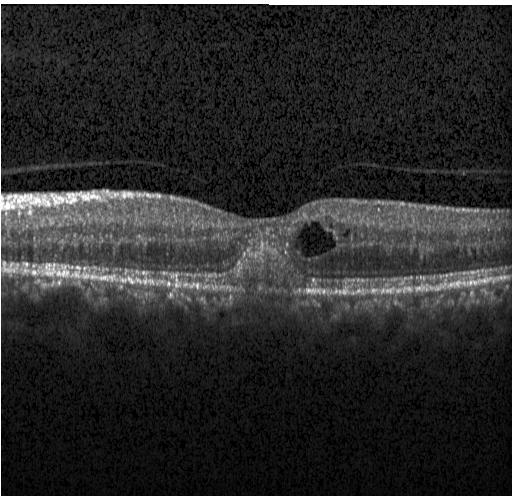 Spectral-domain OCT, fovea-centered, OCT B-scan, acquired on a Heidelberg Spectralis.
A choroidal neovascular membrane.